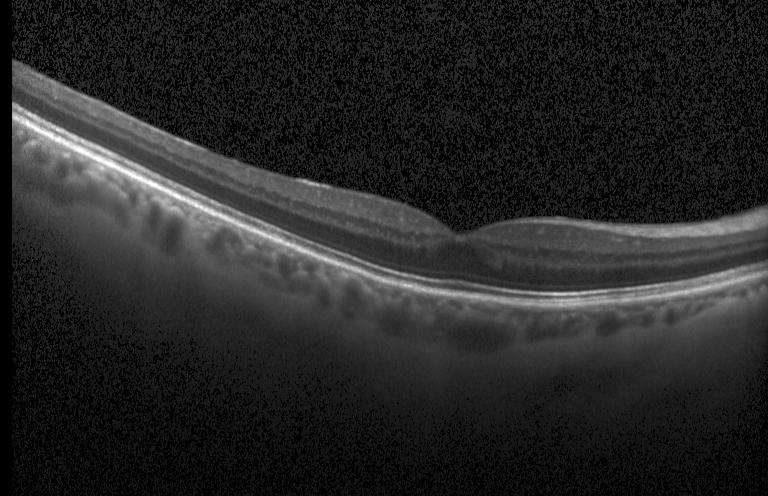

Dx: no evidence of choroidal neovascularization, diabetic macular edema, or drusen.